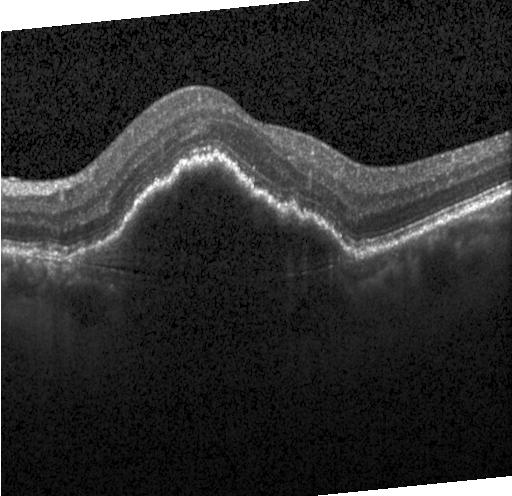

OCT finding: choroidal neovascularization.